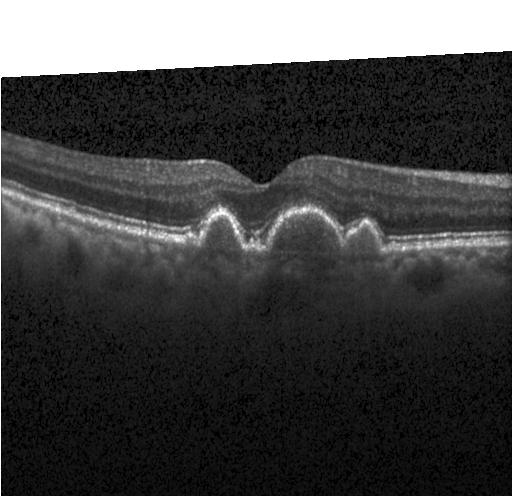
Macular scan; acquired on a Heidelberg Spectralis; spectral-domain optical coherence tomography; OCT B-scan — The scan shows multiple drusen.